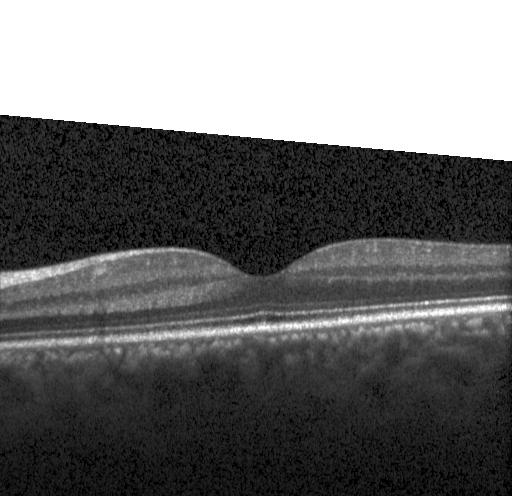

Retinal OCT B-scan. Centered on the fovea. Heidelberg Spectralis OCT system. Diagnosis: no CNV, no DME, and no drusen.